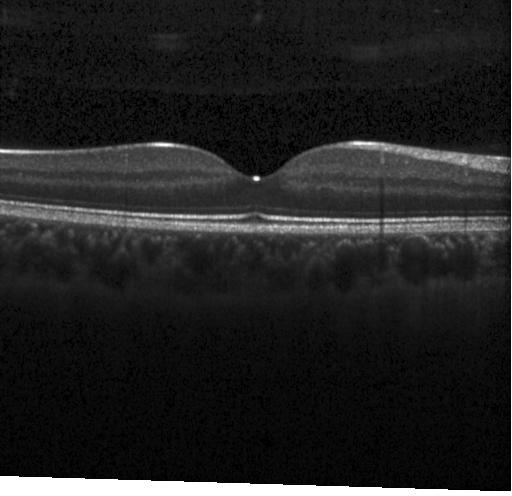

Heidelberg Spectralis OCT system, fovea-centered, SD-OCT, retinal OCT B-scan. The scan shows no CNV, no DME, and no drusen.